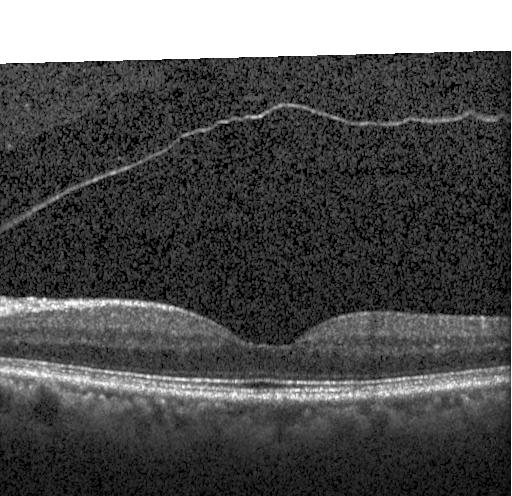
Instrument: Heidelberg Spectralis · optical coherence tomography scan. Impression: no CNV, no DME, and no drusen.